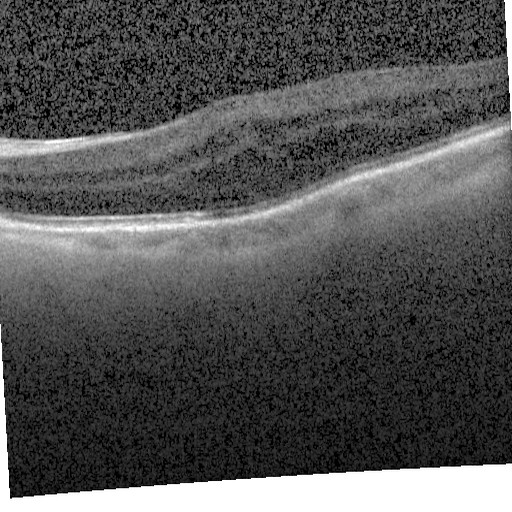
Diagnosis: diabetic macular edema (DME).